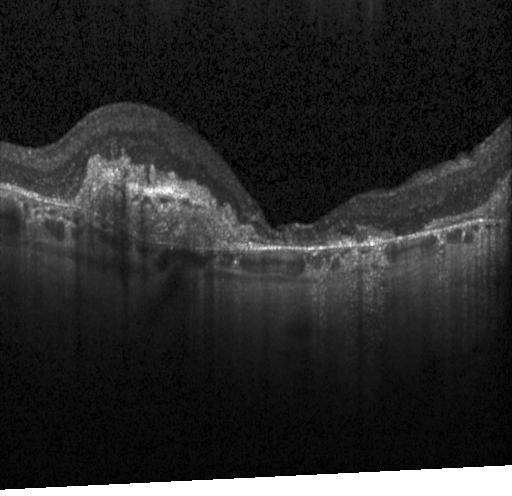
OCT finding: choroidal neovascularization (CNV).